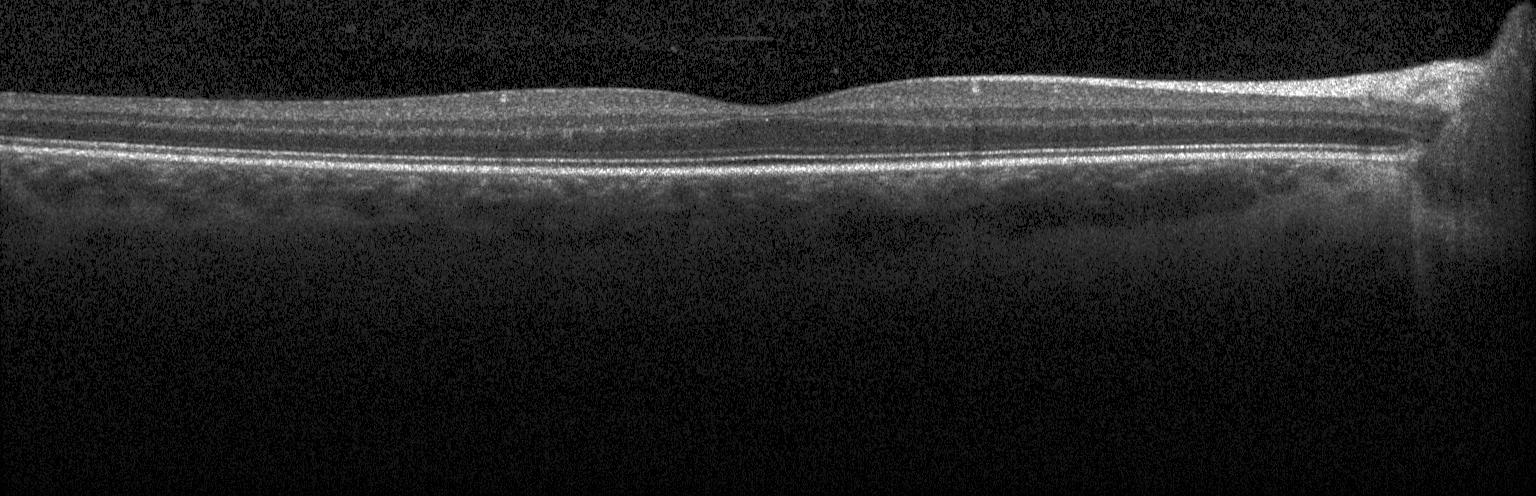 OCT B-scan. Spectral-domain optical coherence tomography.
Finding: no CNV, no DME, and no drusen.